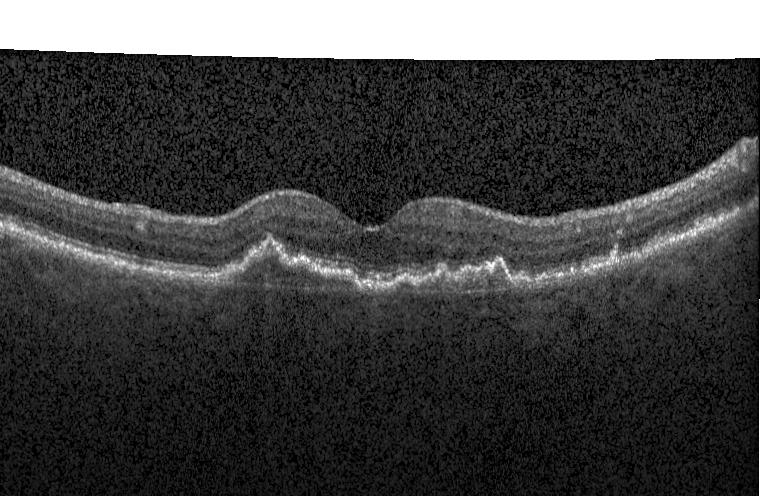 Optical coherence tomography B-scan, spectral-domain OCT
Diagnosis: a choroidal neovascular membrane.